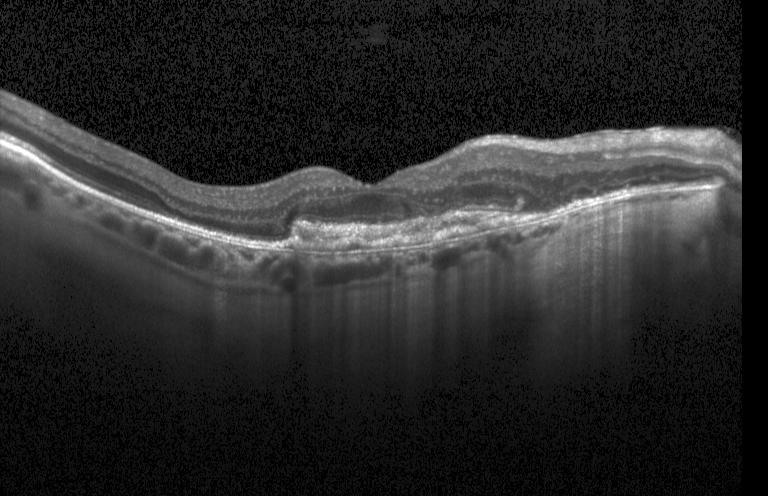
Dx: CNV.